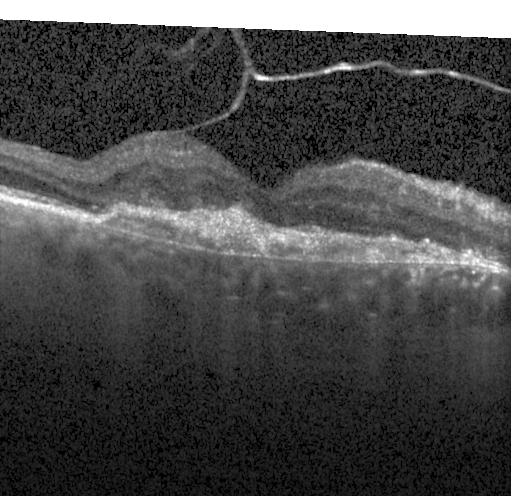 Retinal OCT B-scan, through the macula, SD-OCT, acquired on a Heidelberg Spectralis — This B-scan demonstrates choroidal neovascularization.